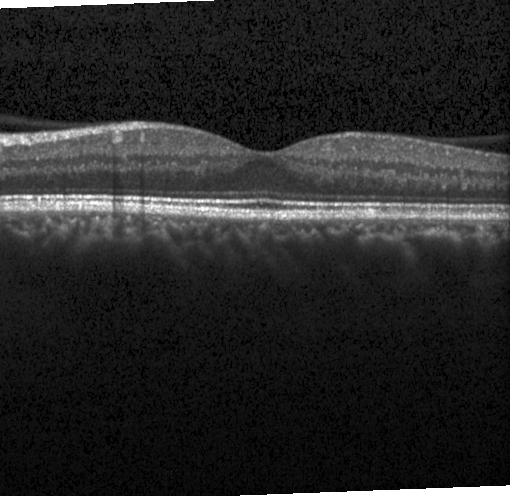

Macular OCT demonstrating neither CNV, DME, nor drusen.